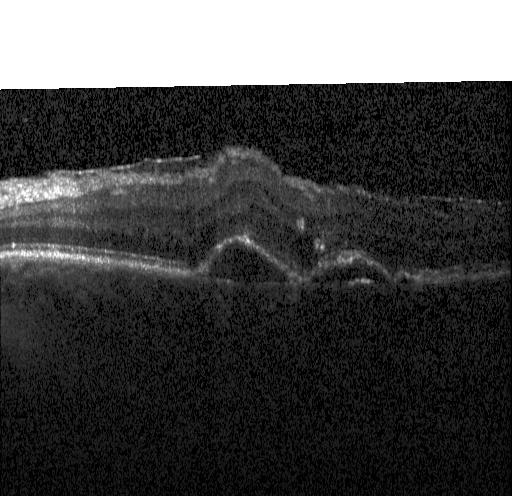 The scan shows CNV.